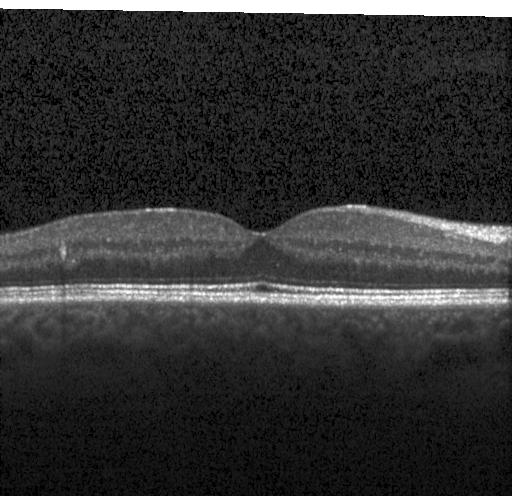 Retinal OCT B-scan; macular scan; spectral-domain OCT. Finding: no choroidal neovascularization, no diabetic macular edema, and no drusen.